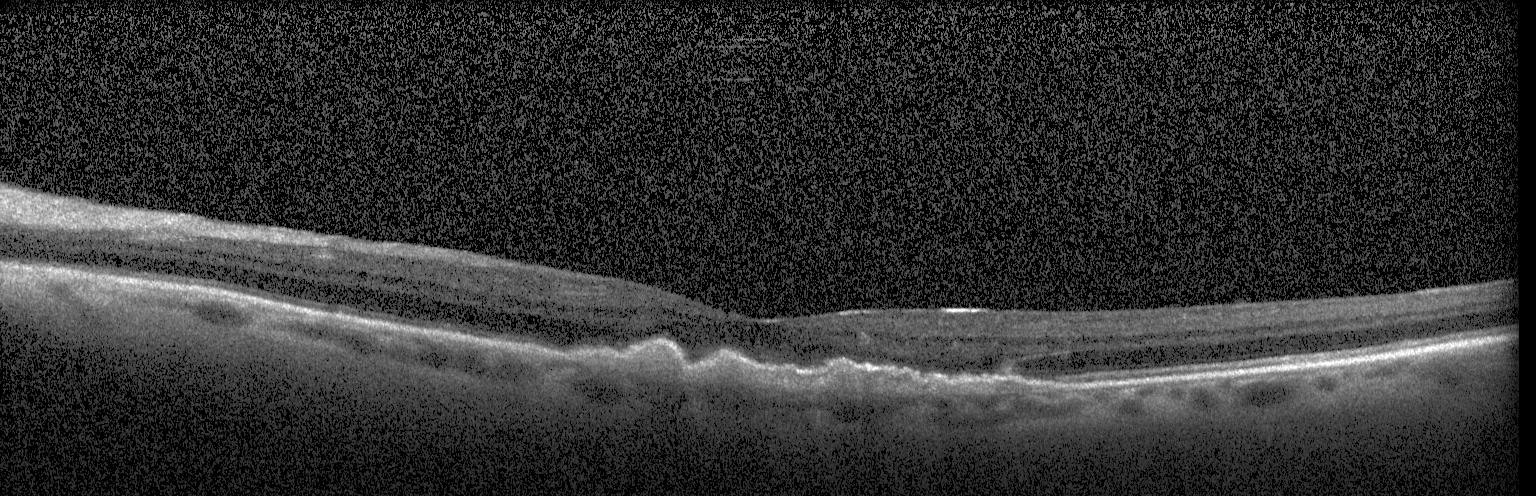

Retinal OCT B-scan · Heidelberg Spectralis · centered on the fovea · spectral-domain OCT
Diagnosis: multiple drusen.